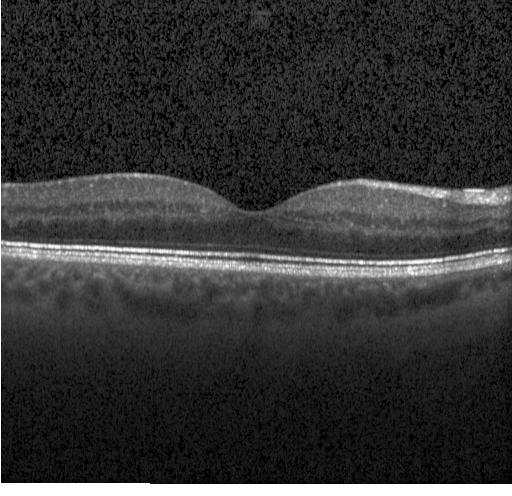

Optical coherence tomography scan.
No choroidal neovascularization, diabetic macular edema, or drusen.